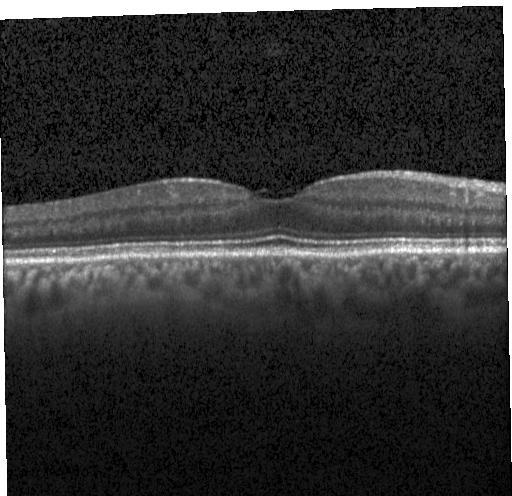 OCT scan showing no CNV, no DME, and no drusen.